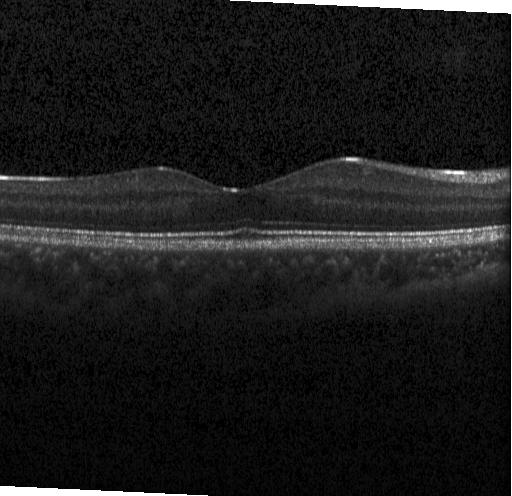
Heidelberg Spectralis OCT system. Fovea-centered. Spectral-domain optical coherence tomography. Retinal OCT cross-section.
Dx: neither choroidal neovascularization, diabetic macular edema, nor drusen.